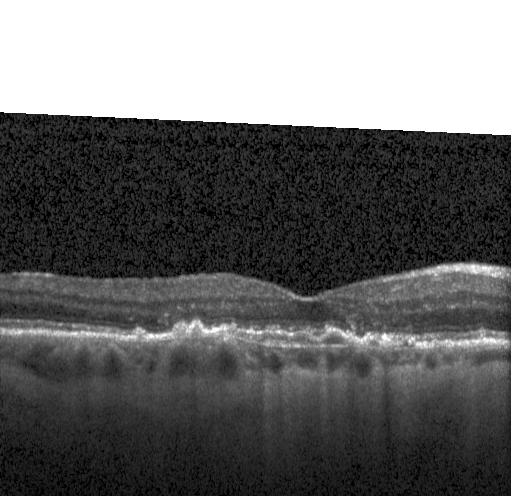
Optical coherence tomography B-scan, instrument: Heidelberg Spectralis, horizontal scan through the fovea. Finding: a choroidal neovascular membrane.